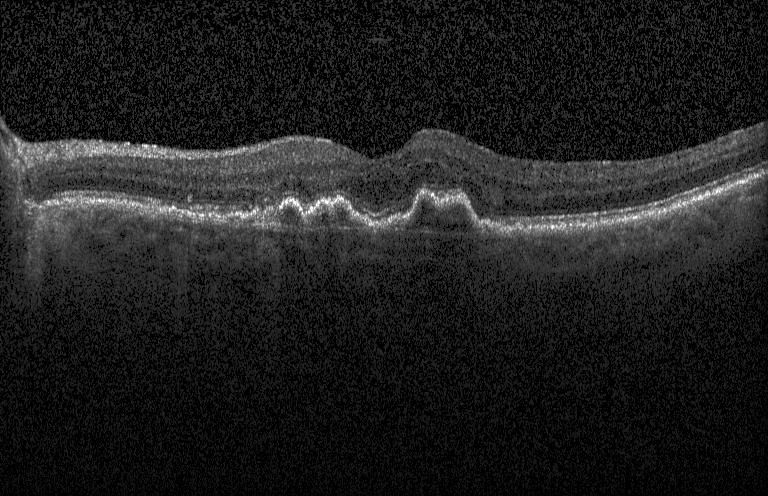 OCT B-scan — This B-scan demonstrates a choroidal neovascular membrane.